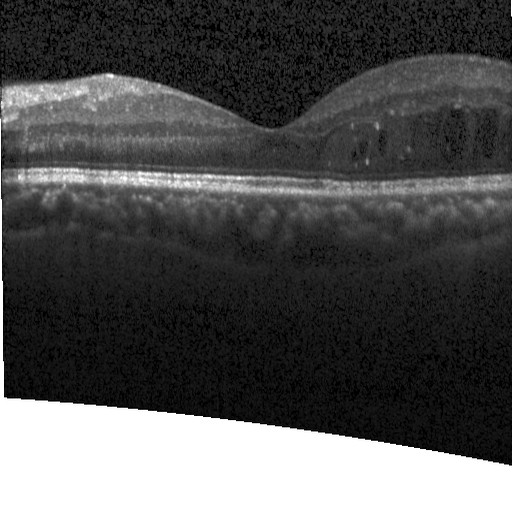 OCT line scan
Impression: DME.